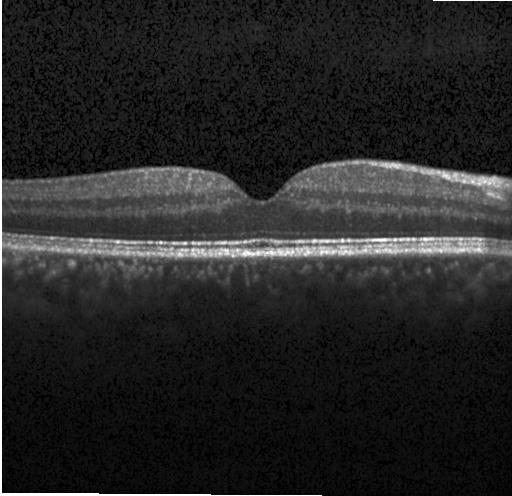
Retinal OCT cross-section · Heidelberg Spectralis OCT system · macular scan
This B-scan demonstrates neither CNV, DME, nor drusen.